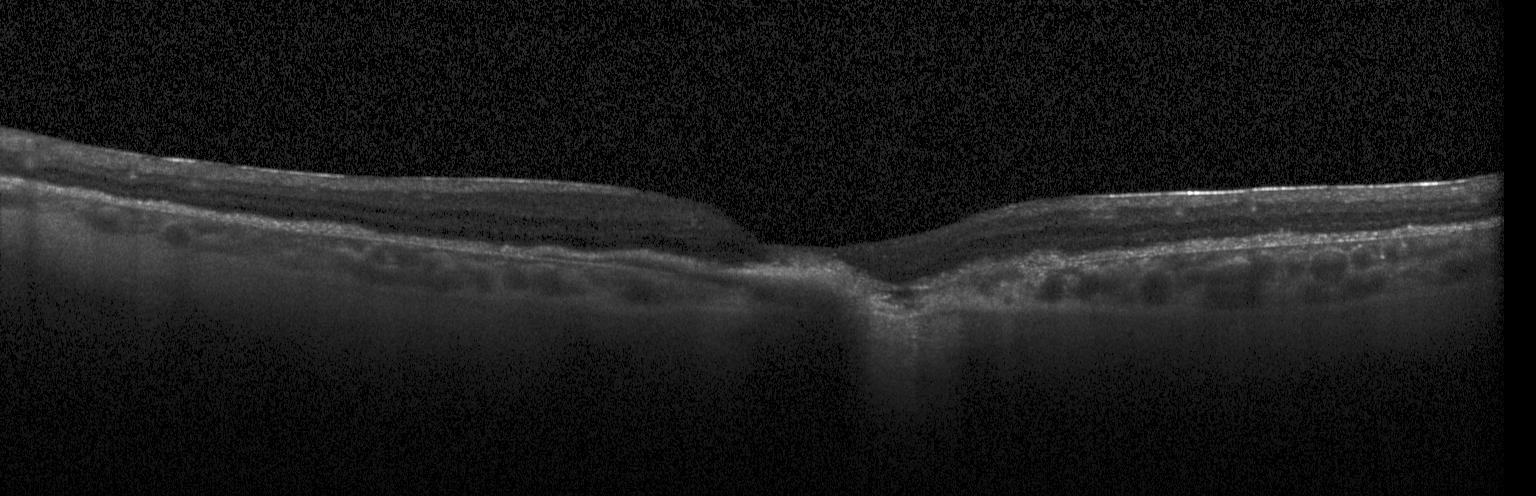 Optical coherence tomography B-scan; Heidelberg Spectralis; SD-OCT; fovea-centered
This B-scan demonstrates choroidal neovascularization (CNV).